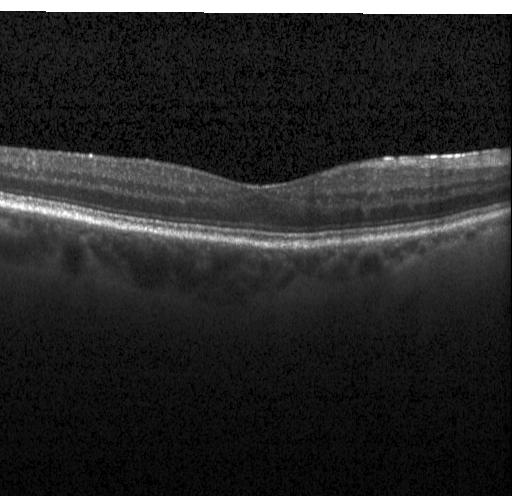
Optical coherence tomography scan, acquired on a Heidelberg Spectralis — Diagnosis: no choroidal neovascularization, no diabetic macular edema, and no drusen.